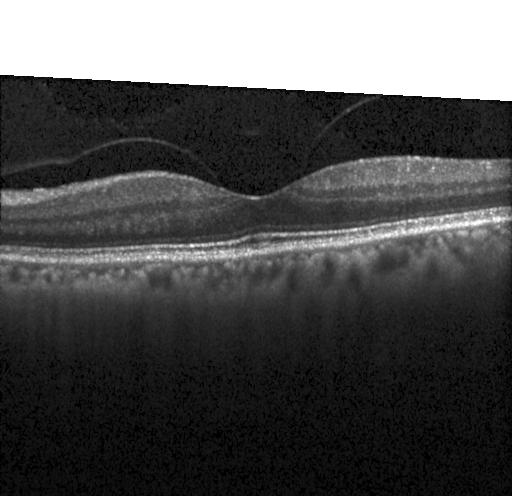
Spectral-domain OCT, OCT line scan, Heidelberg Spectralis OCT system
Diagnosis: neither choroidal neovascularization, diabetic macular edema, nor drusen.